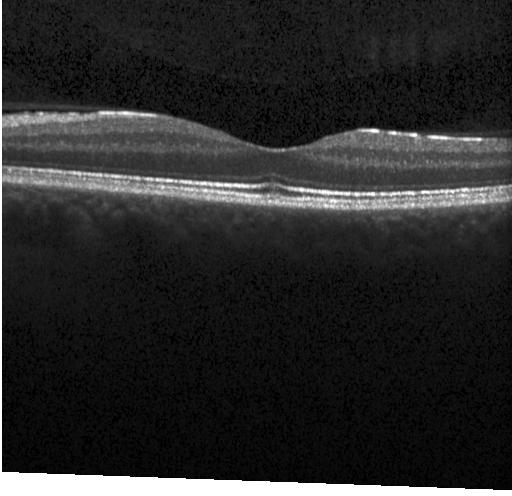
This B-scan demonstrates no choroidal neovascularization, no diabetic macular edema, and no drusen.